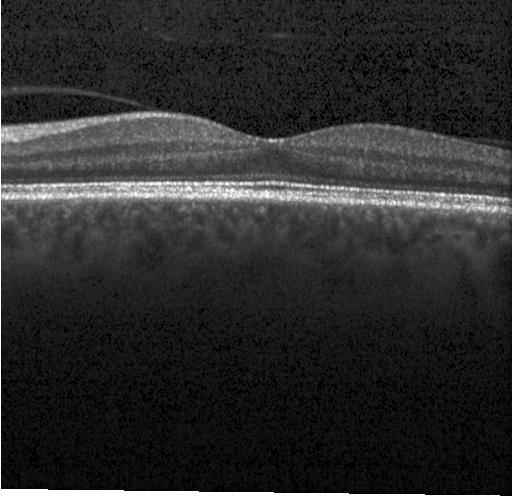
Finding: no choroidal neovascularization, no diabetic macular edema, and no drusen.